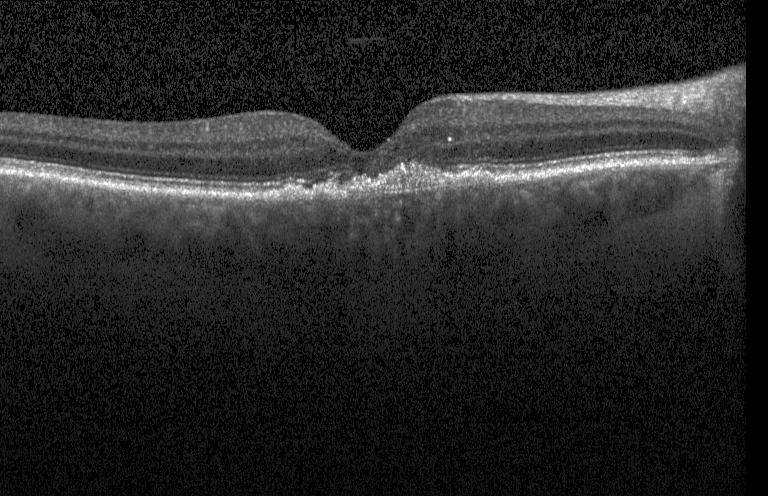
OCT line scan — Assessment: CNV.